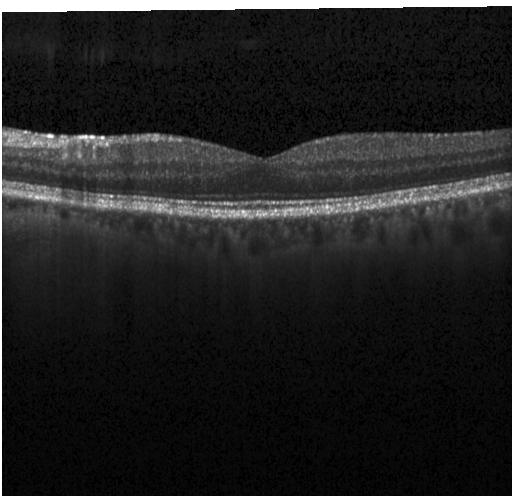
Through the macula, spectral-domain optical coherence tomography, OCT B-scan, Heidelberg Spectralis OCT system.
Macular OCT: neither choroidal neovascularization, diabetic macular edema, nor drusen.